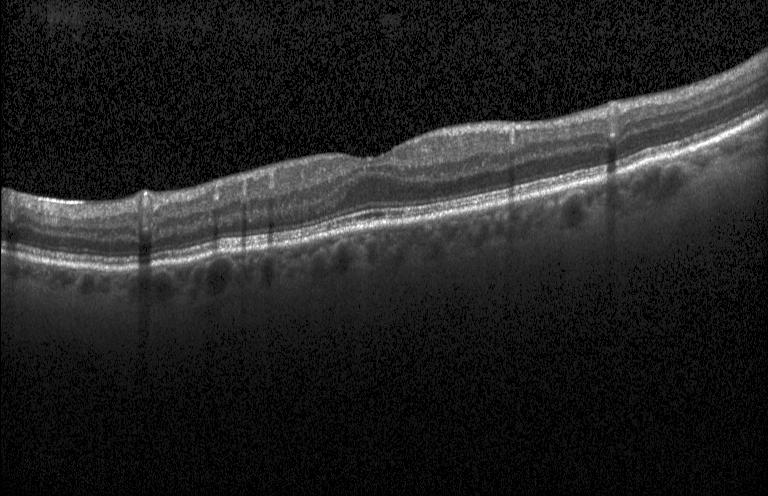
Optical coherence tomography scan. Fovea-centered. SD-OCT. Acquired on a Heidelberg Spectralis
No evidence of choroidal neovascularization, diabetic macular edema, or drusen.